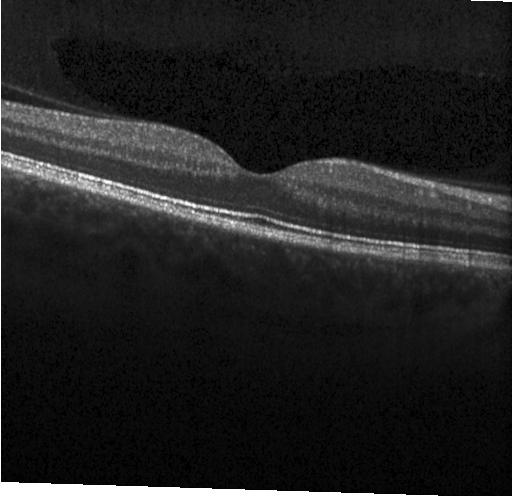
Fovea-centered, optical coherence tomography B-scan, SD-OCT.
Impression: no choroidal neovascularization, no diabetic macular edema, and no drusen.